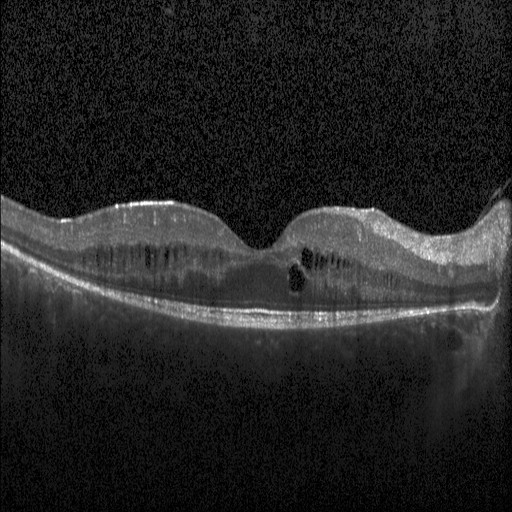 Macular OCT: DME.